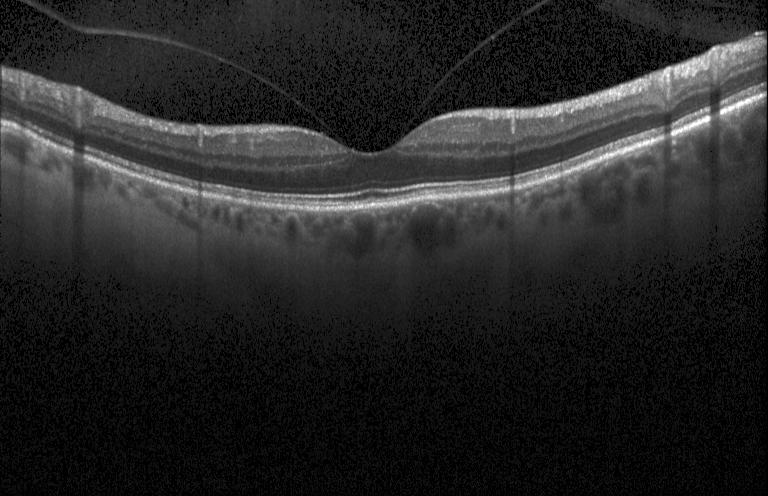
Optical coherence tomography B-scan.
Impression: no choroidal neovascularization, diabetic macular edema, or drusen.